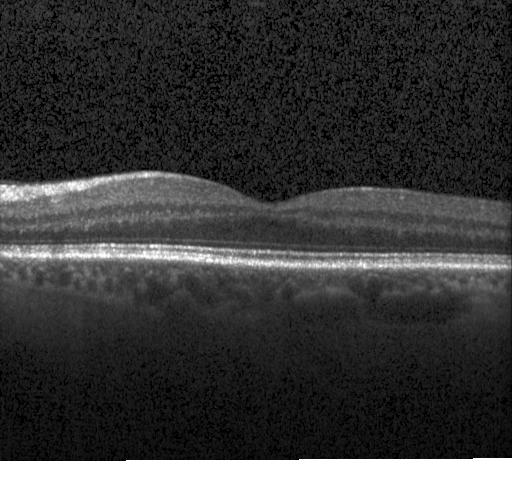

OCT finding: no choroidal neovascularization, no diabetic macular edema, and no drusen.